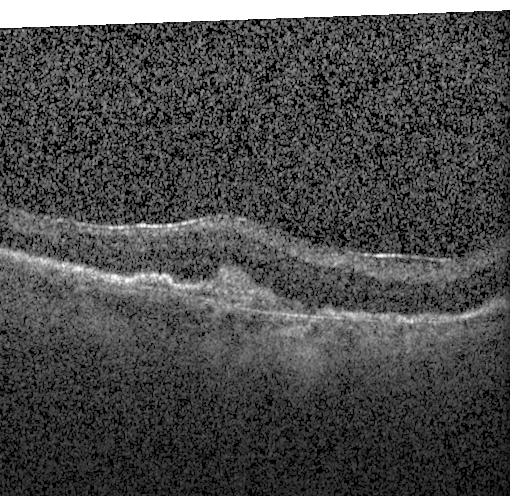

Instrument: Heidelberg Spectralis. Optical coherence tomography scan — Dx: a choroidal neovascular membrane.